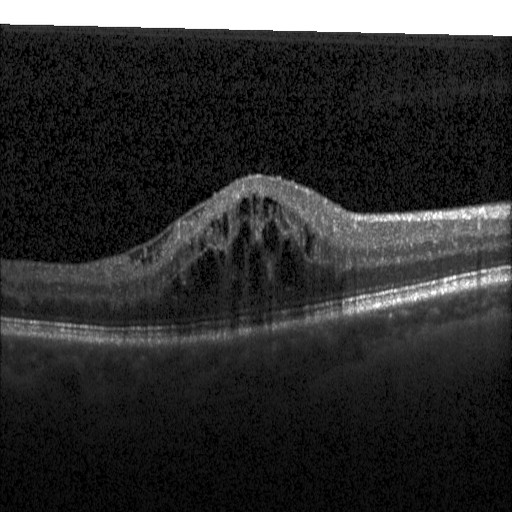
Retinal OCT cross-section — This B-scan demonstrates diabetic macular edema (DME).